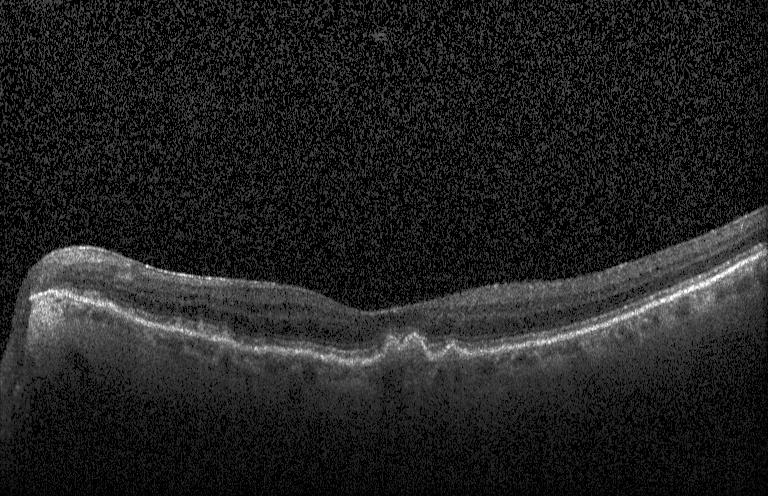

Centered on the fovea. SD-OCT. Optical coherence tomography scan. Sub-RPE drusenoid deposits.